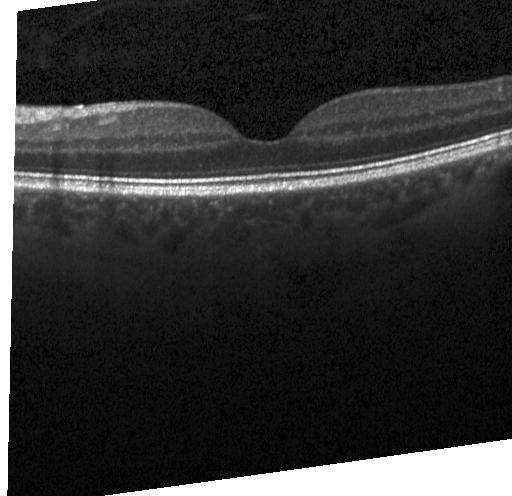

Heidelberg Spectralis OCT system; retinal OCT cross-section
Finding: no choroidal neovascularization, diabetic macular edema, or drusen.